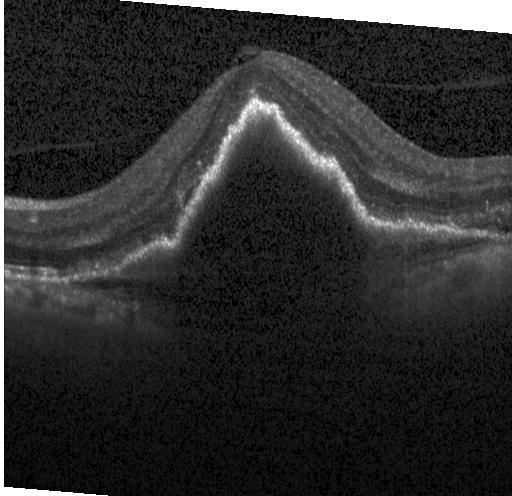

Impression: choroidal neovascularization (CNV).